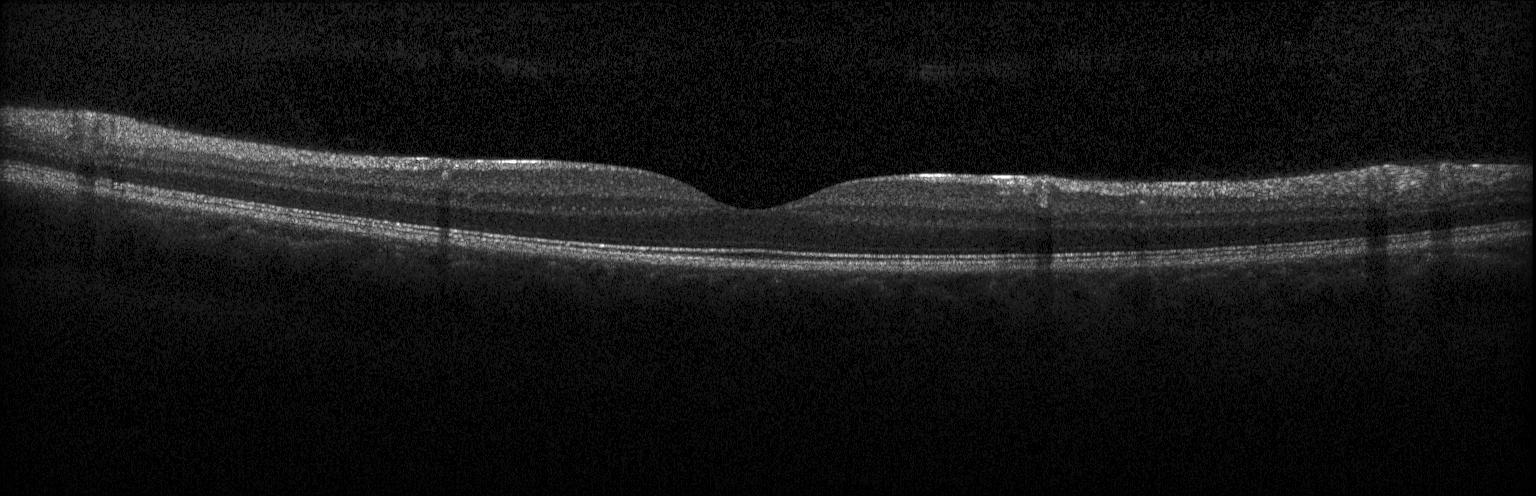

Macular scan. Optical coherence tomography scan. Spectral-domain OCT. Macular OCT: neither choroidal neovascularization, diabetic macular edema, nor drusen.